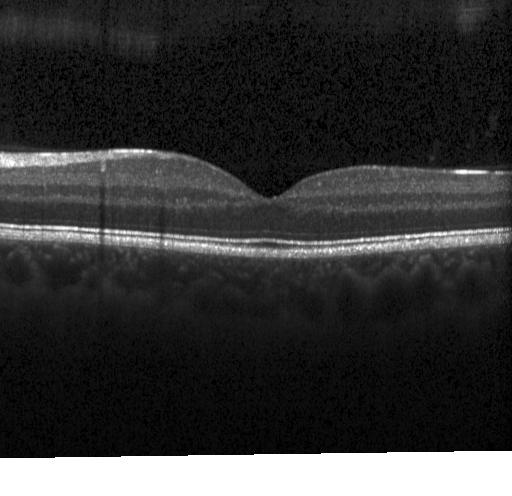

This B-scan demonstrates no evidence of choroidal neovascularization, diabetic macular edema, or drusen.